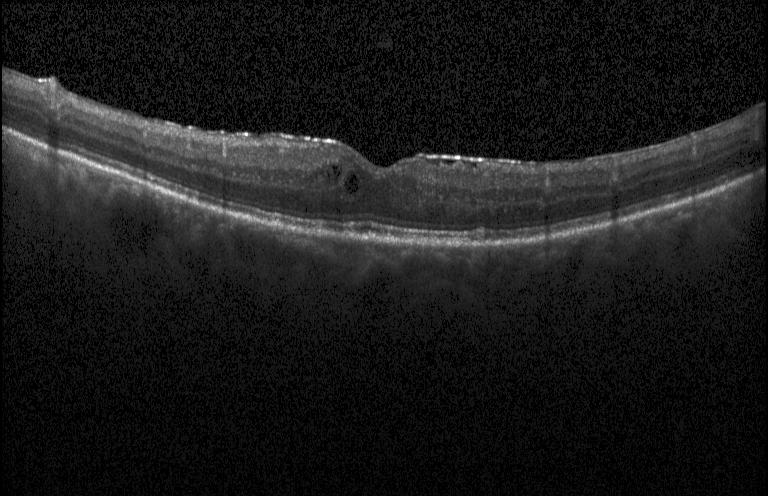
Macular scan; spectral-domain OCT; instrument: Heidelberg Spectralis; retinal OCT cross-section — The scan shows DME.